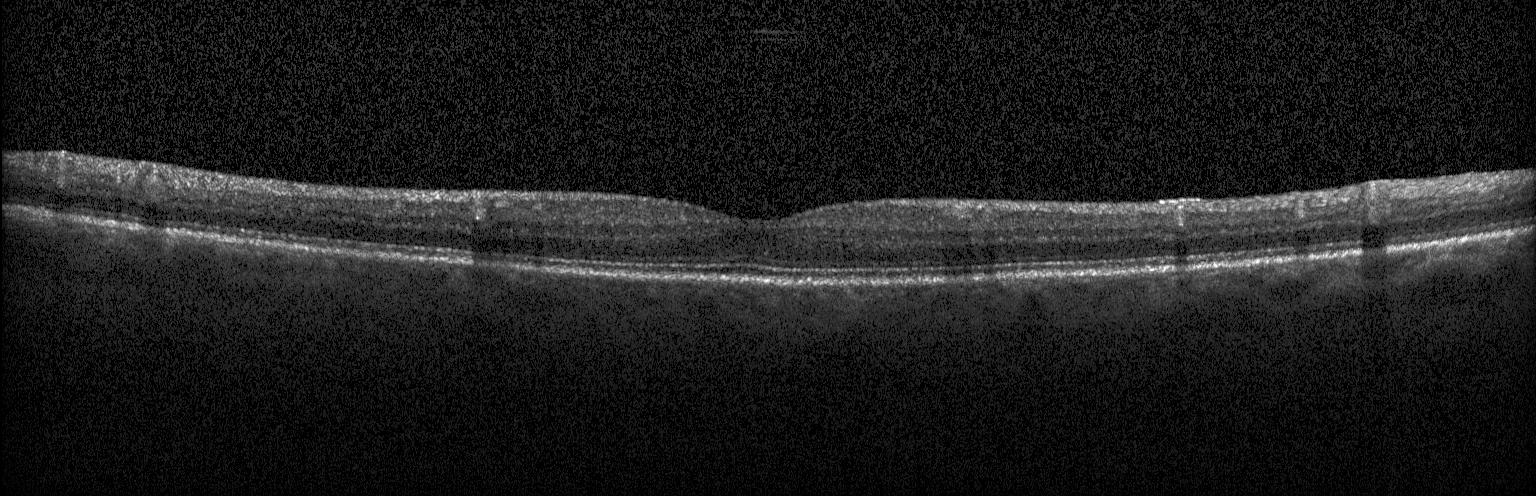
OCT B-scan — Diagnosis: neither choroidal neovascularization, diabetic macular edema, nor drusen.